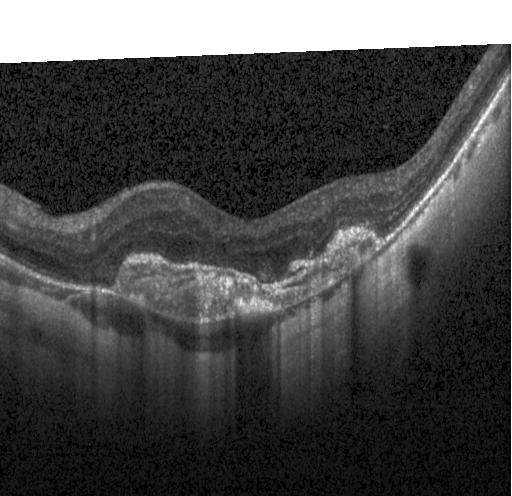 Finding: a choroidal neovascular membrane.